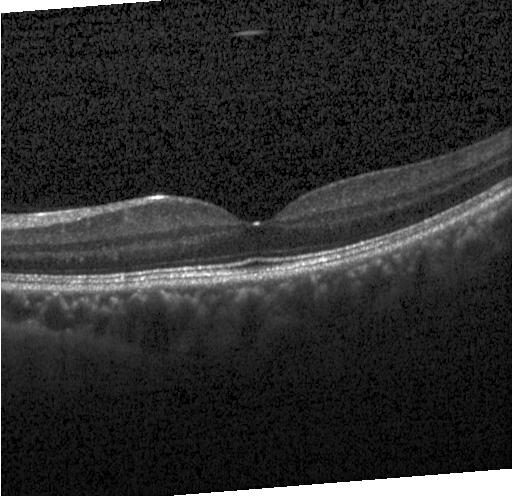

Optical coherence tomography B-scan
Finding: no CNV, no DME, and no drusen.